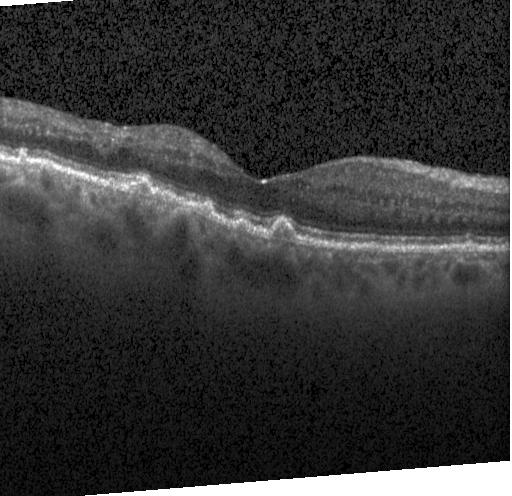 SD-OCT; retinal OCT cross-section.
The scan shows multiple drusen.